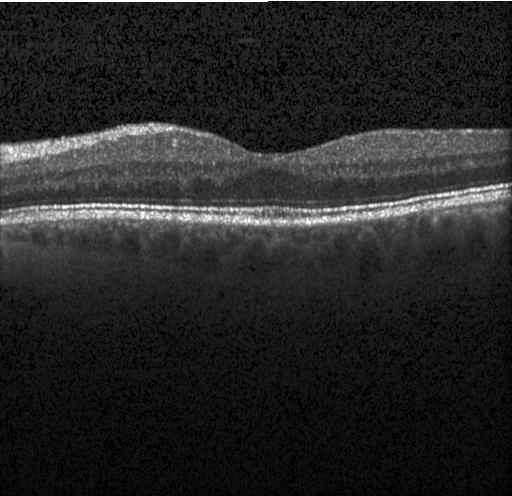 Macular OCT: neither choroidal neovascularization, diabetic macular edema, nor drusen.